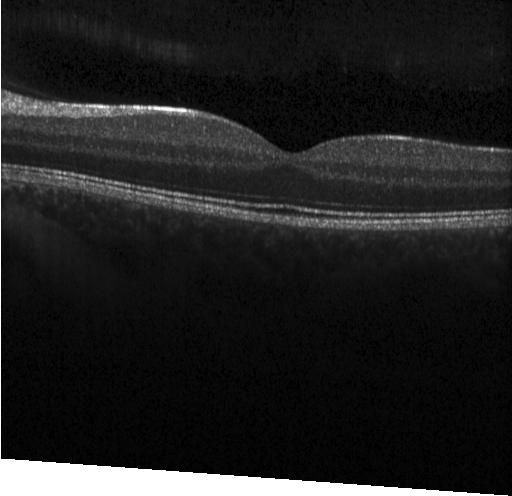
OCT B-scan · horizontal scan through the fovea · spectral-domain optical coherence tomography.
Finding: no CNV, no DME, and no drusen.